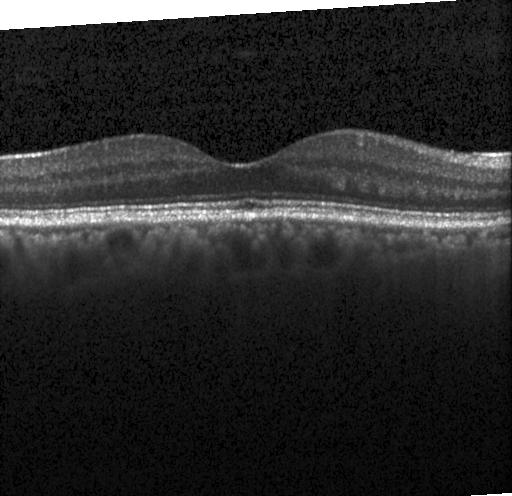

OCT B-scan; Heidelberg Spectralis; spectral-domain OCT. Diagnosis: neither choroidal neovascularization, diabetic macular edema, nor drusen.